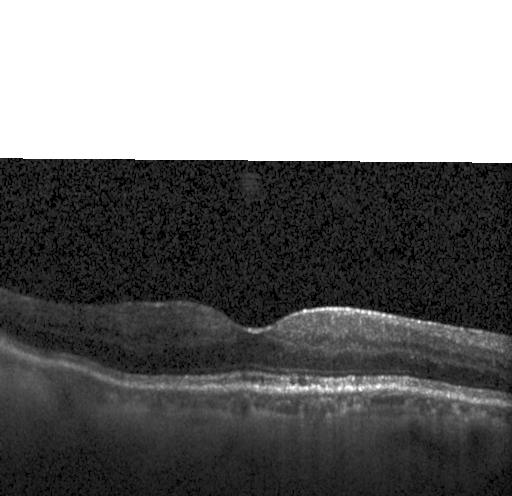

Centered on the fovea. Acquired on a Heidelberg Spectralis. OCT B-scan — Diagnosis: no CNV, DME, or drusen.